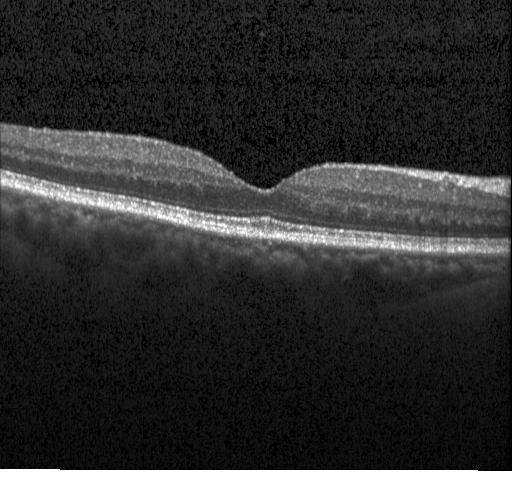 Optical coherence tomography scan. Spectral-domain optical coherence tomography
The scan shows no choroidal neovascularization, diabetic macular edema, or drusen.